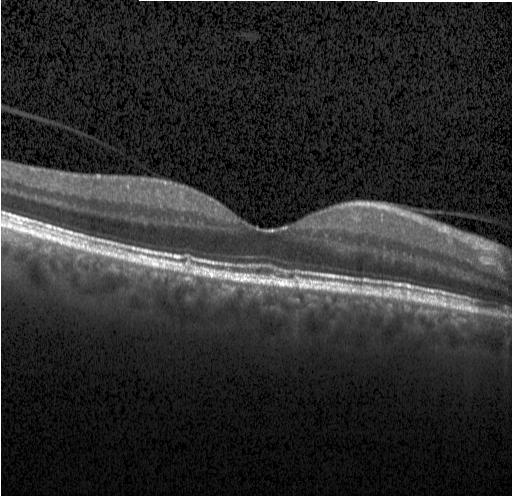

Macular OCT: drusen.